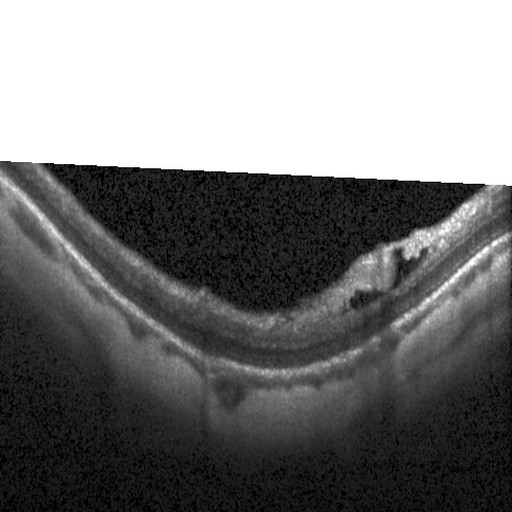

This B-scan demonstrates diabetic macular edema.